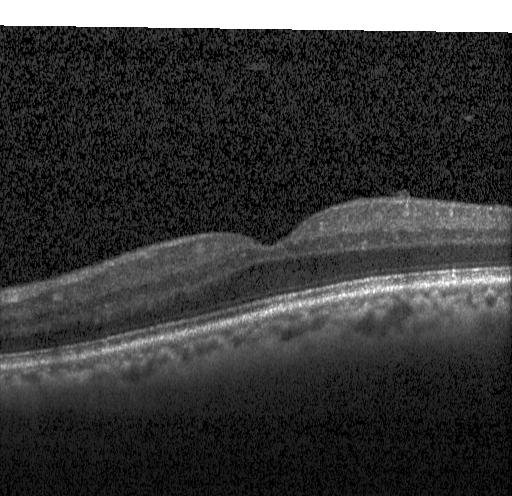
The scan shows no CNV, no DME, and no drusen.